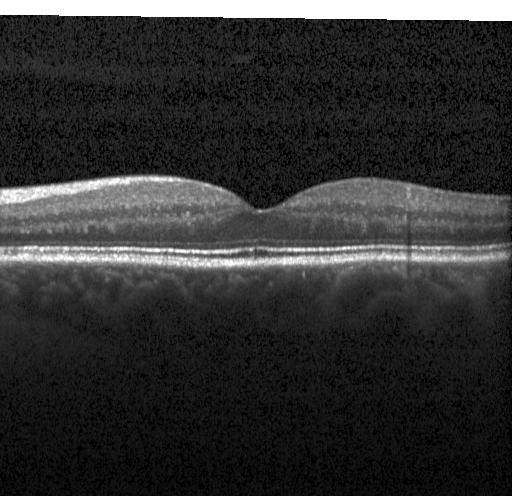
Impression: neither choroidal neovascularization, diabetic macular edema, nor drusen.